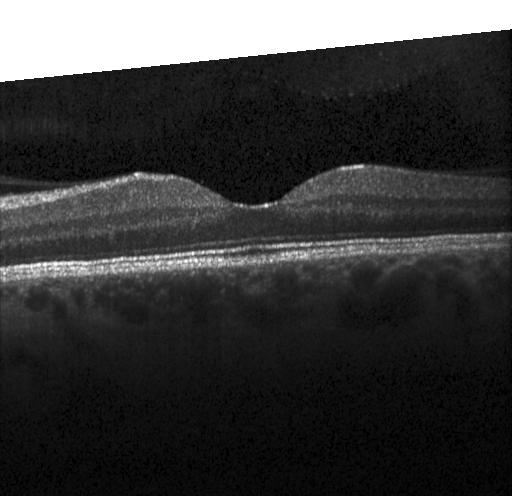

Diagnosis: no evidence of choroidal neovascularization, diabetic macular edema, or drusen.